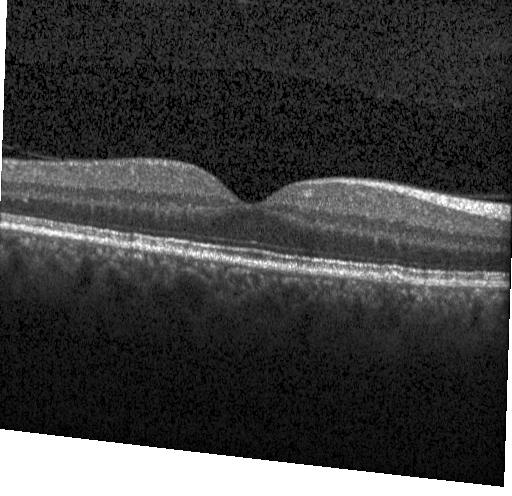 Neither CNV, DME, nor drusen.